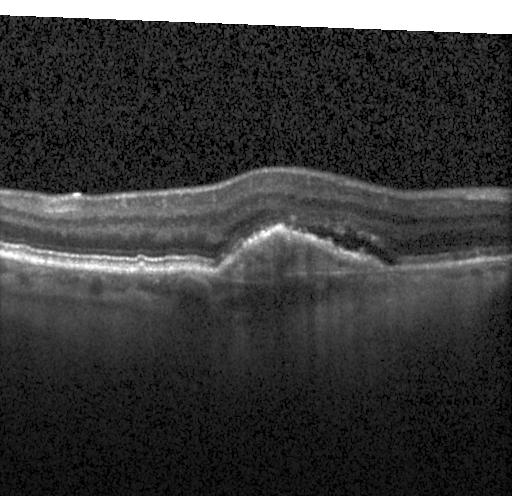
Centered on the fovea. Retinal OCT B-scan. Instrument: Heidelberg Spectralis. SD-OCT. Assessment: choroidal neovascularization (CNV).